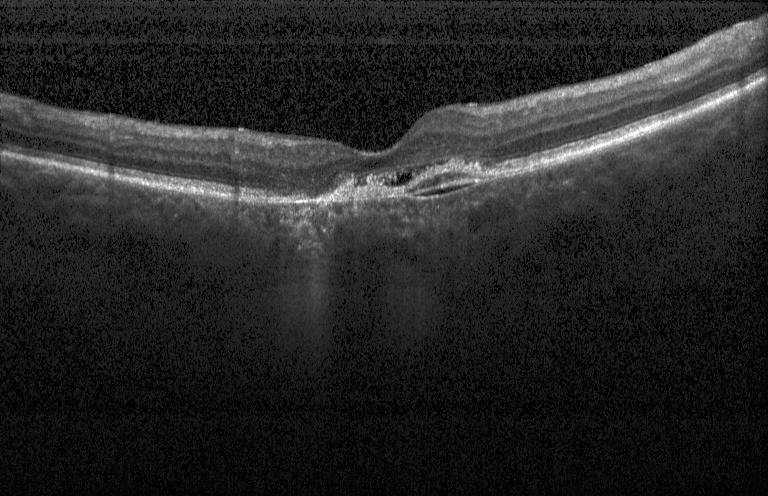
OCT line scan — This B-scan demonstrates choroidal neovascularization (CNV).